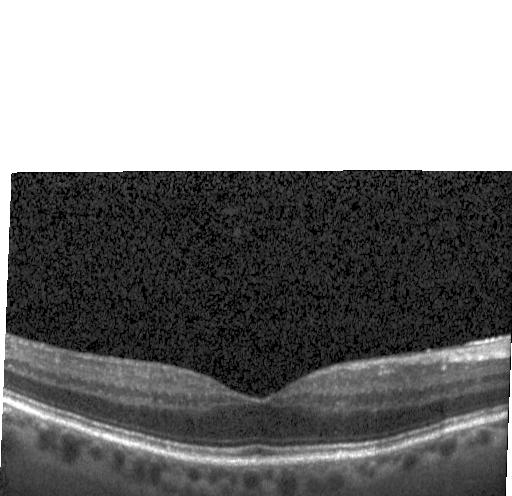
Retinal OCT cross-section showing no choroidal neovascularization, diabetic macular edema, or drusen.